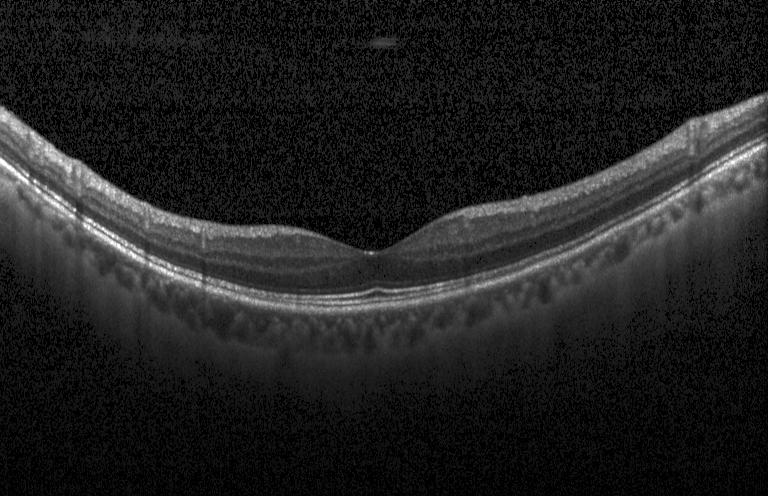
Assessment: no choroidal neovascularization, diabetic macular edema, or drusen.